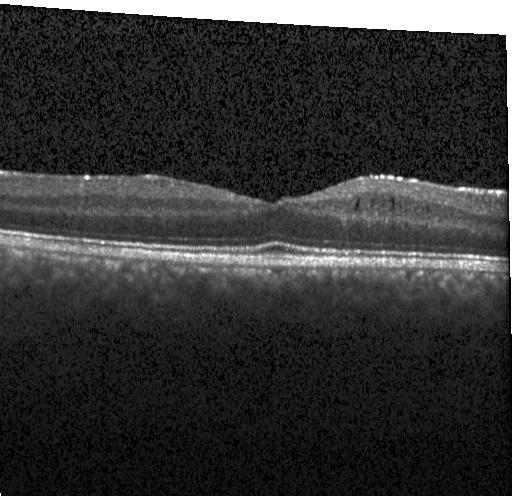

Optical coherence tomography scan, Heidelberg Spectralis, centered on the fovea. Finding: diabetic macular edema.